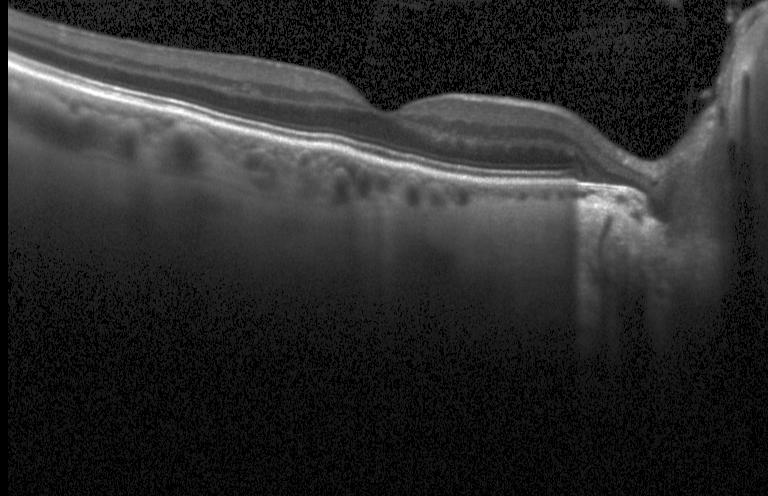 Finding: no evidence of CNV, DME, or drusen.